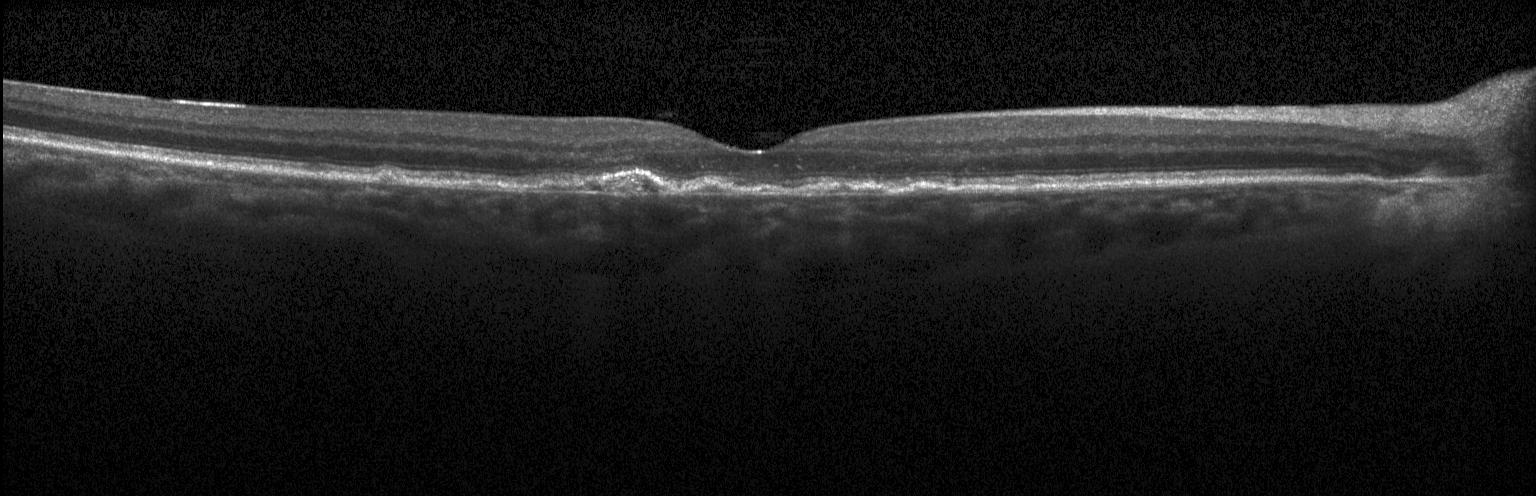

OCT scan showing a choroidal neovascular membrane.